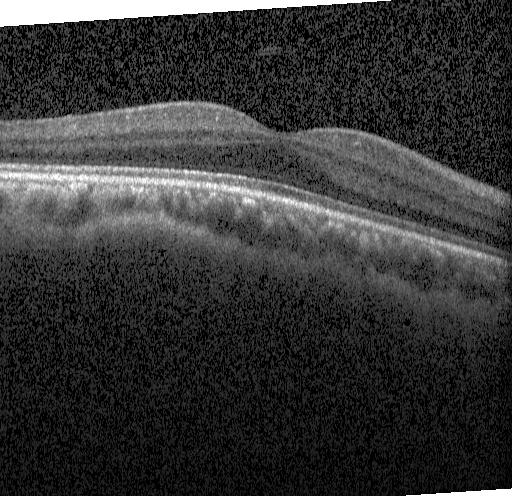
No evidence of choroidal neovascularization, diabetic macular edema, or drusen.